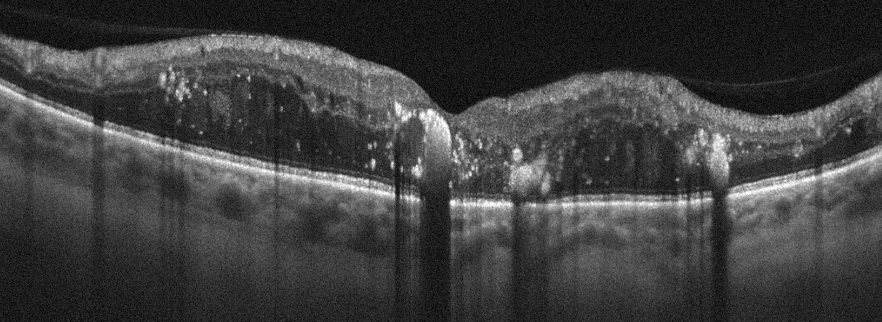

Optovue Avanti RTVue XR, optical coherence tomography B-scan. OCT finding: diabetic macular edema.